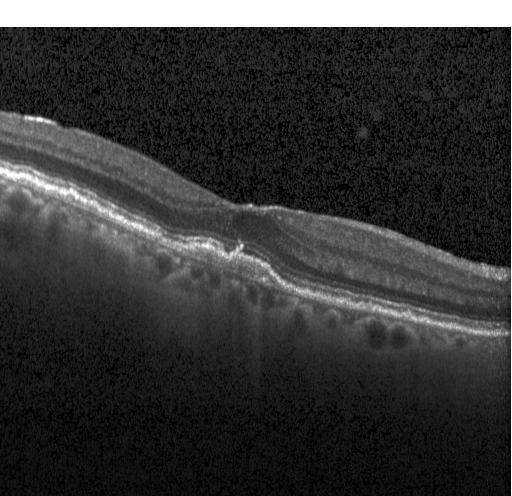
Impression: choroidal neovascularization.